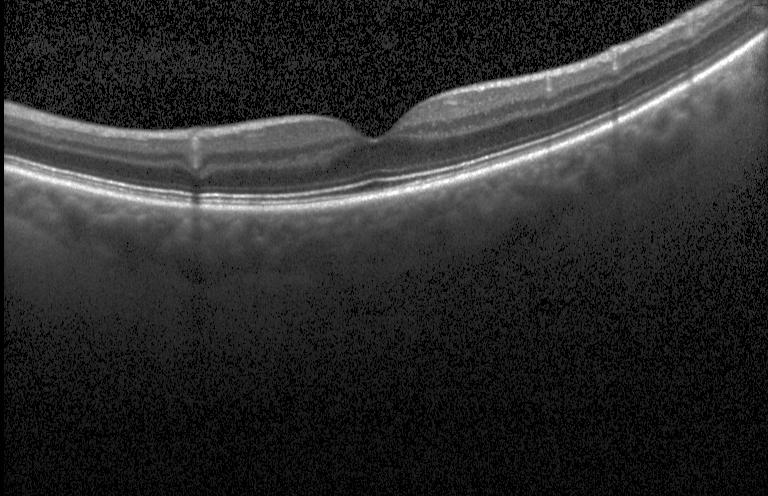
Retinal OCT B-scan — Dx: neither choroidal neovascularization, diabetic macular edema, nor drusen.